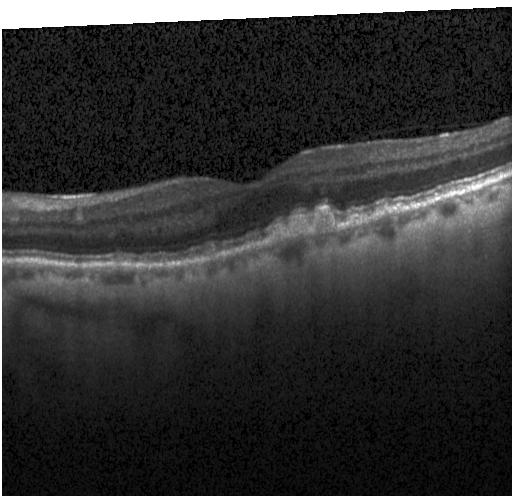
Finding: sub-RPE drusenoid deposits.